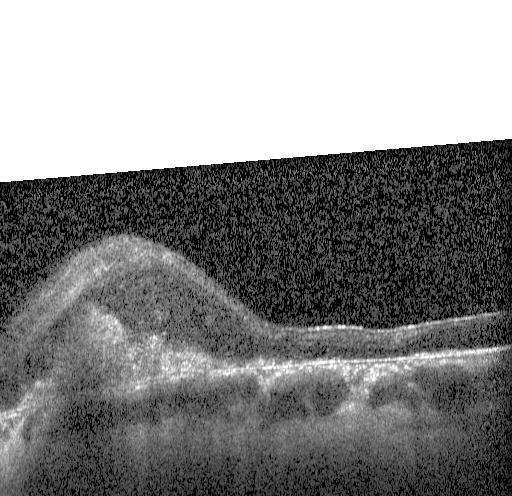

Spectral-domain OCT B-scan: a choroidal neovascular membrane.